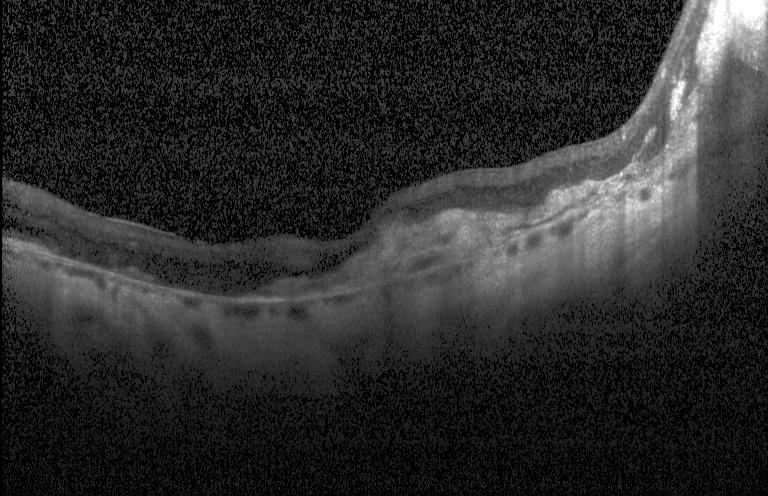
Heidelberg Spectralis, macular scan, SD-OCT, optical coherence tomography B-scan.
Assessment: a choroidal neovascular membrane.